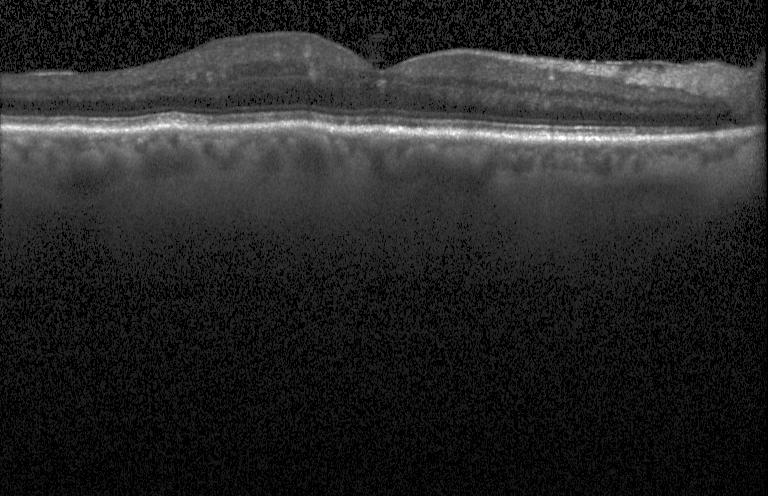

Optical coherence tomography scan.
No choroidal neovascularization, diabetic macular edema, or drusen.